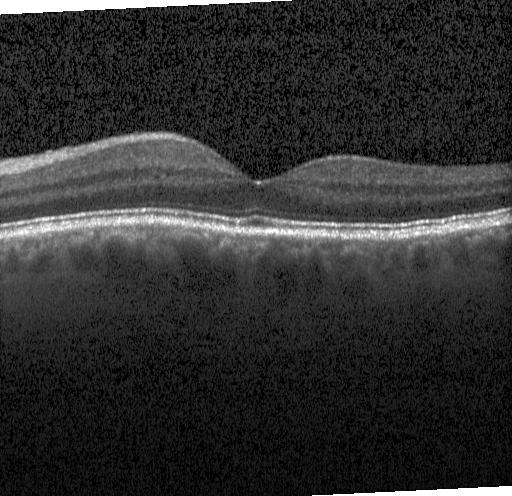 OCT line scan.
Impression: no choroidal neovascularization, diabetic macular edema, or drusen.